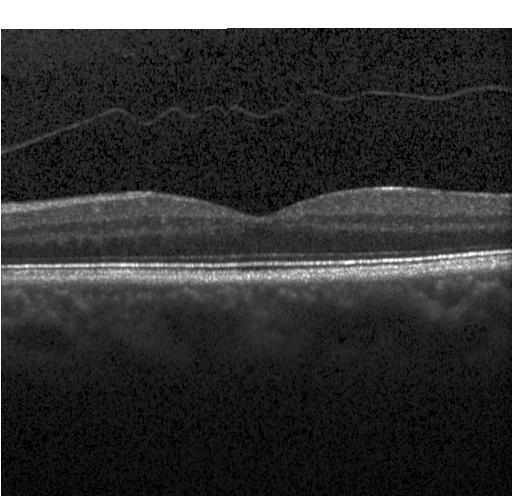
SD-OCT. Macular scan. OCT B-scan — This B-scan demonstrates neither choroidal neovascularization, diabetic macular edema, nor drusen.